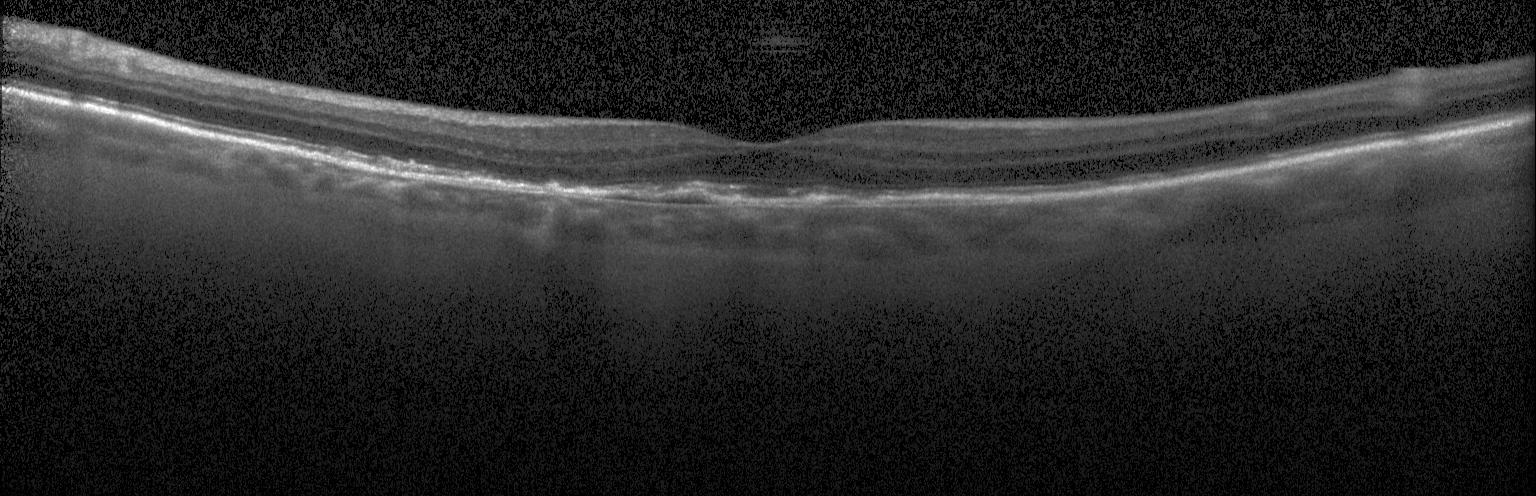
Diagnosis: a choroidal neovascular membrane.